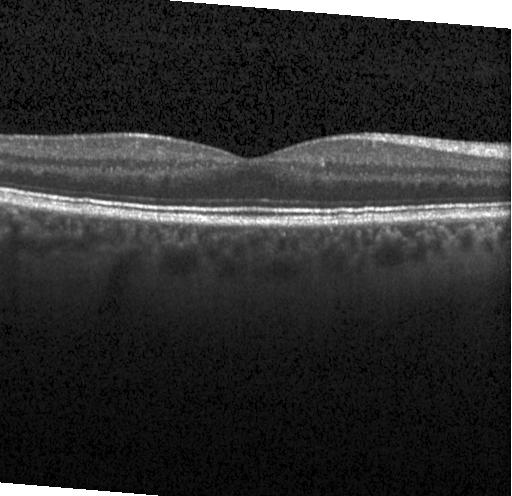

Heidelberg Spectralis, optical coherence tomography B-scan, spectral-domain OCT — This B-scan demonstrates neither CNV, DME, nor drusen.